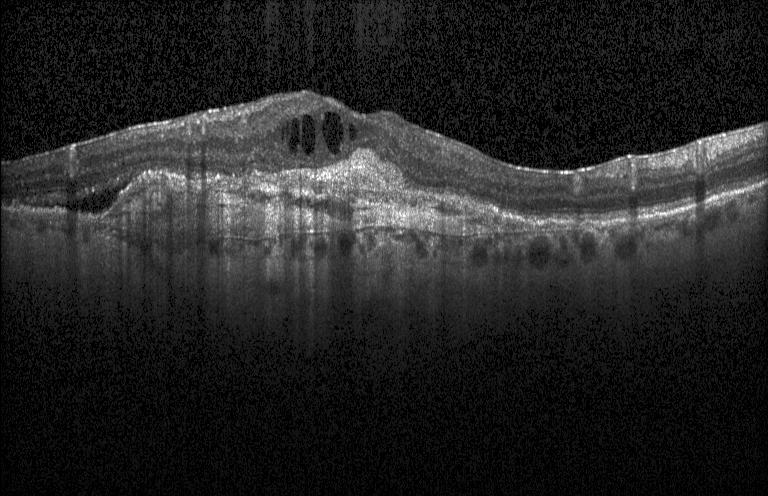 OCT line scan. Instrument: Heidelberg Spectralis — Finding: choroidal neovascularization (CNV).